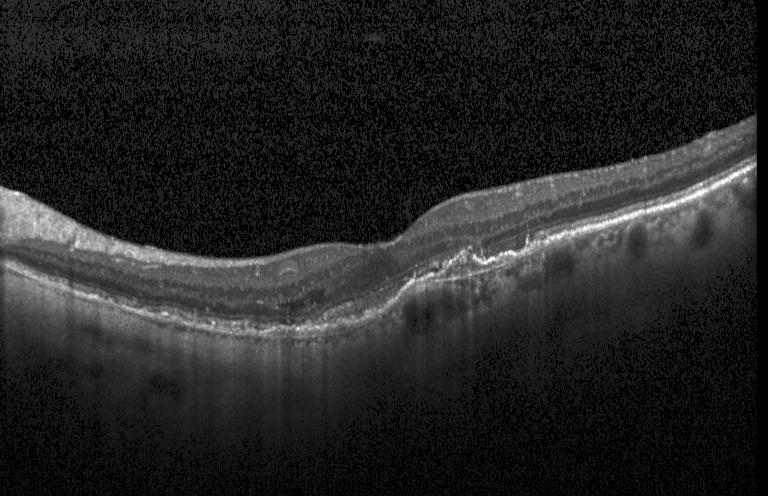
Spectral-domain optical coherence tomography, optical coherence tomography B-scan, acquired on a Heidelberg Spectralis
A choroidal neovascular membrane.